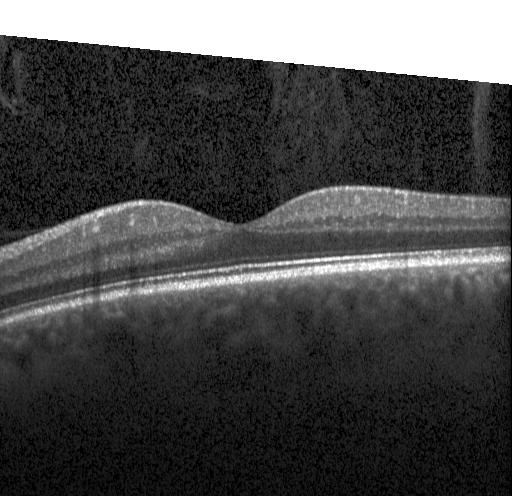 Optical coherence tomography B-scan. Spectral-domain optical coherence tomography
Dx: neither choroidal neovascularization, diabetic macular edema, nor drusen.